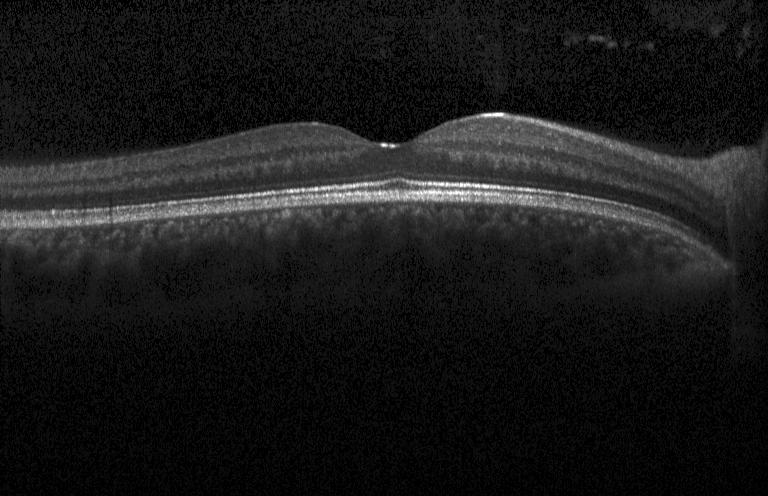 Finding: no CNV, no DME, and no drusen.